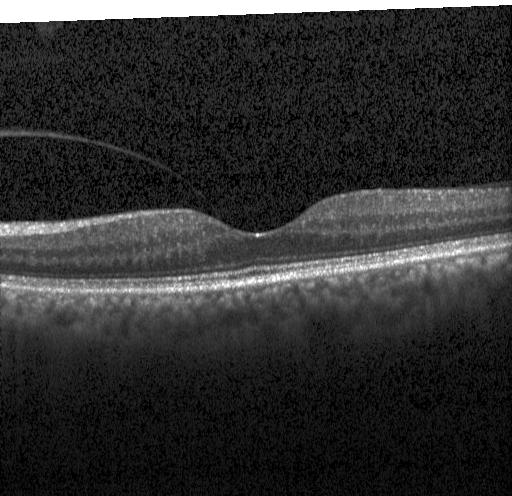

Optical coherence tomography scan.
Impression: no evidence of CNV, DME, or drusen.